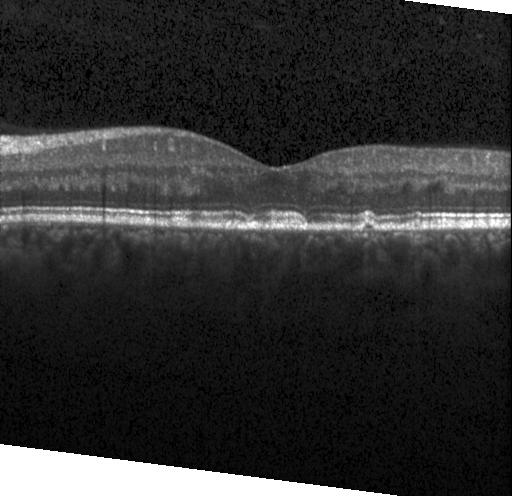
Diagnosis: drusen.